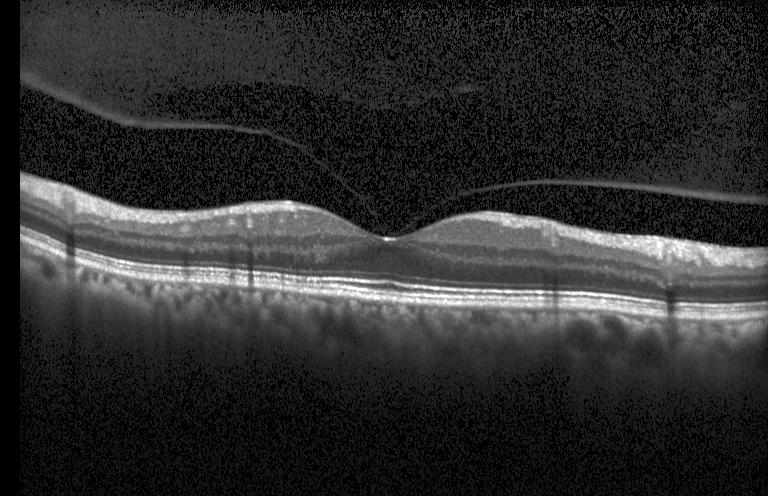 Impression: neither CNV, DME, nor drusen.